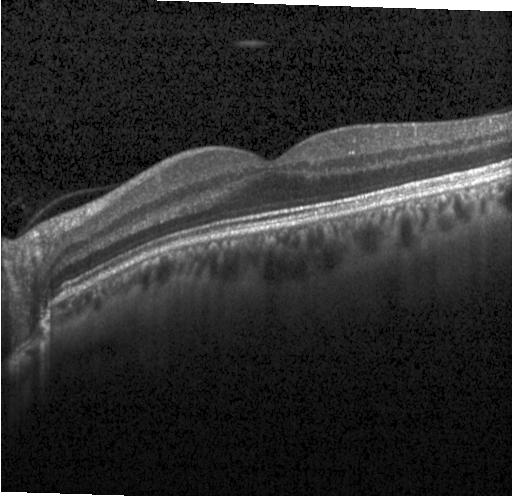

Acquired on a Heidelberg Spectralis, OCT line scan
Finding: no evidence of choroidal neovascularization, diabetic macular edema, or drusen.